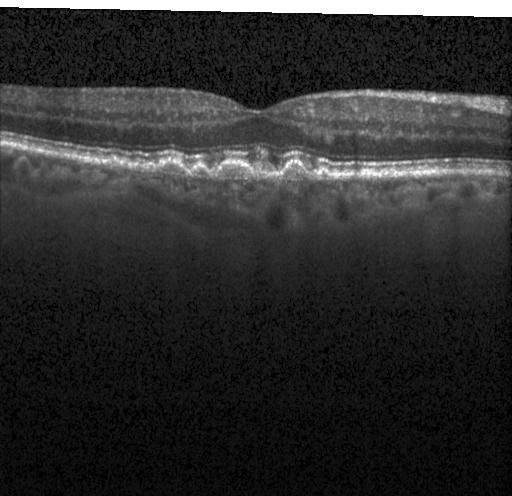 OCT B-scan showing drusen.